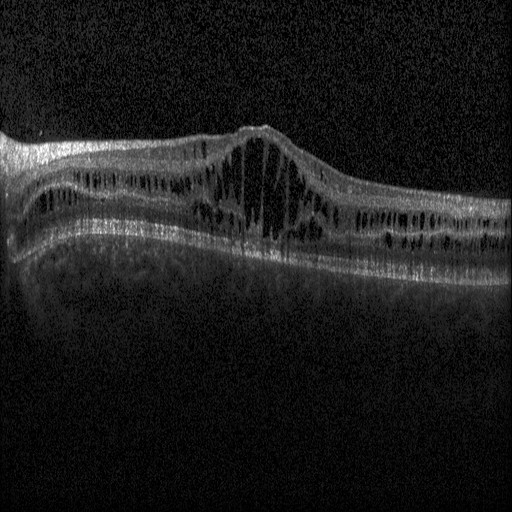 Retinal OCT B-scan
DME.